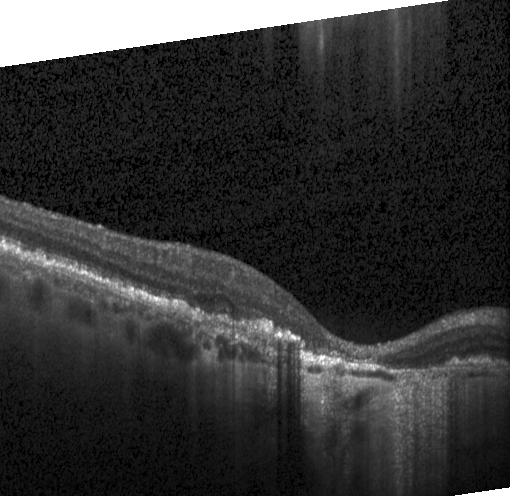

Spectral-domain OCT. Retinal OCT B-scan
This B-scan demonstrates choroidal neovascularization.